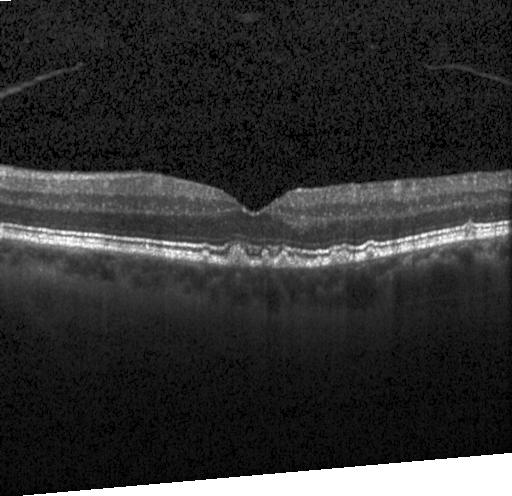 Optical coherence tomography B-scan. Impression: multiple drusen.